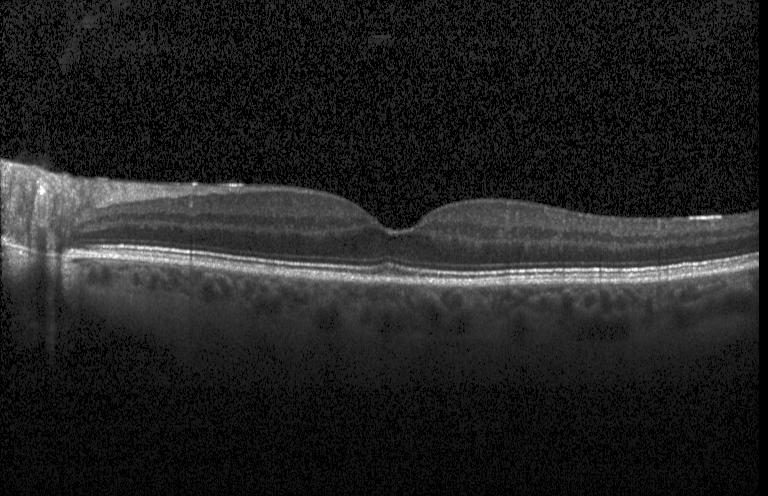
Impression: no CNV, no DME, and no drusen.